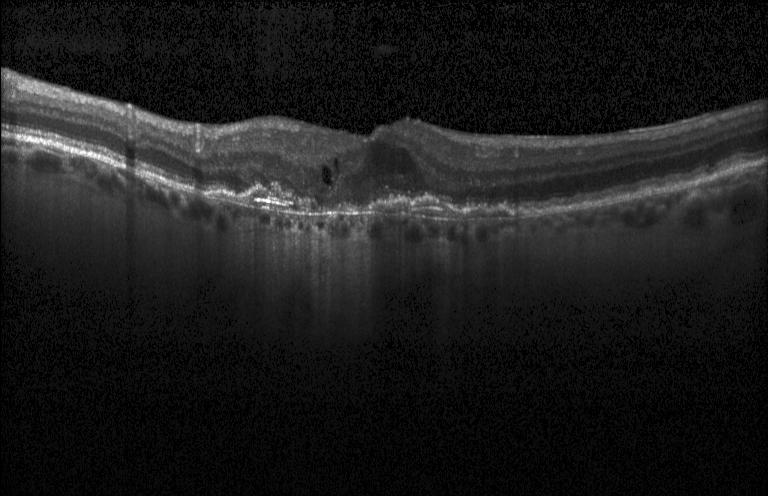
Heidelberg Spectralis OCT system · retinal OCT cross-section
OCT finding: a choroidal neovascular membrane.